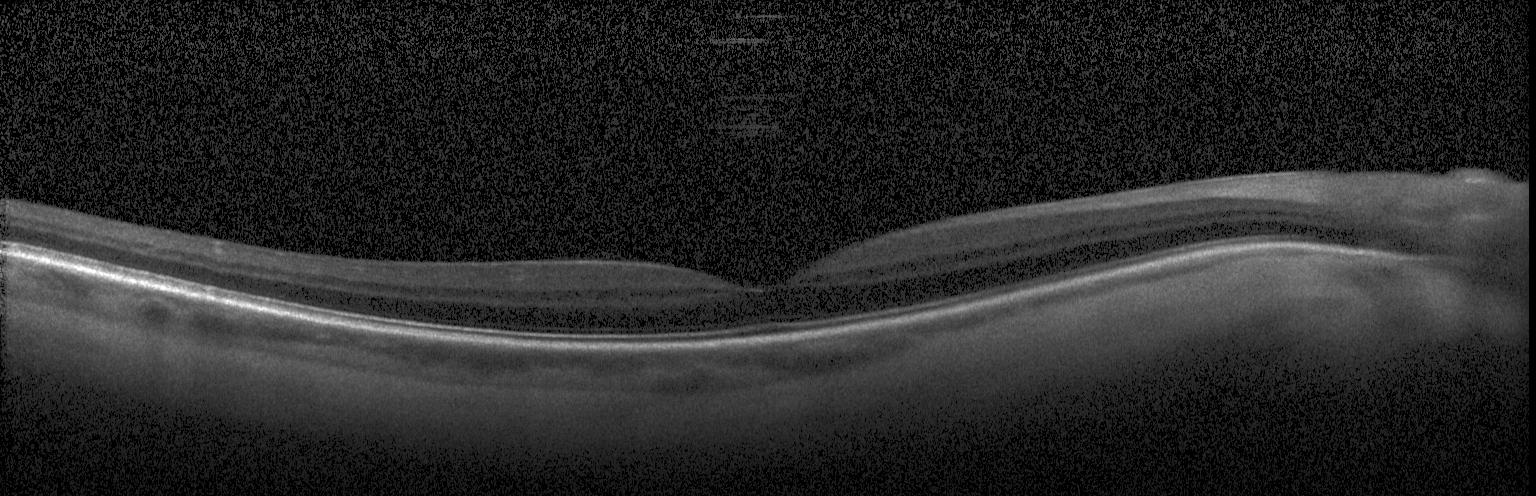
Optical coherence tomography scan · SD-OCT.
This B-scan demonstrates neither choroidal neovascularization, diabetic macular edema, nor drusen.